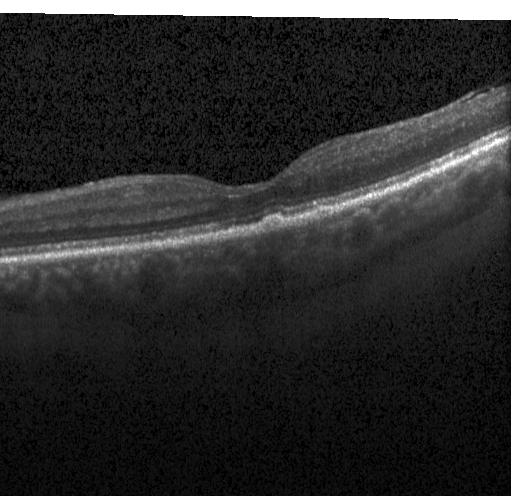 Assessment: sub-RPE drusenoid deposits.